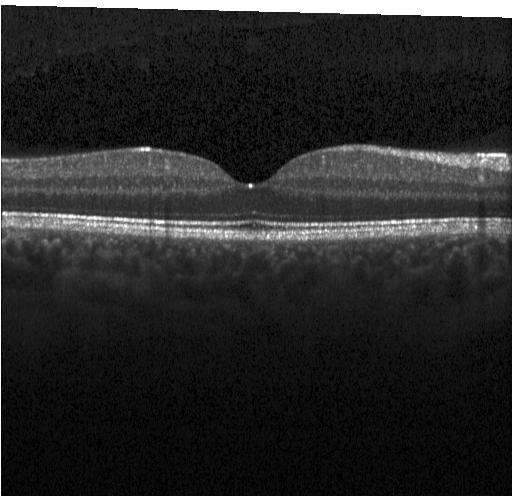

Dx: no CNV, DME, or drusen.